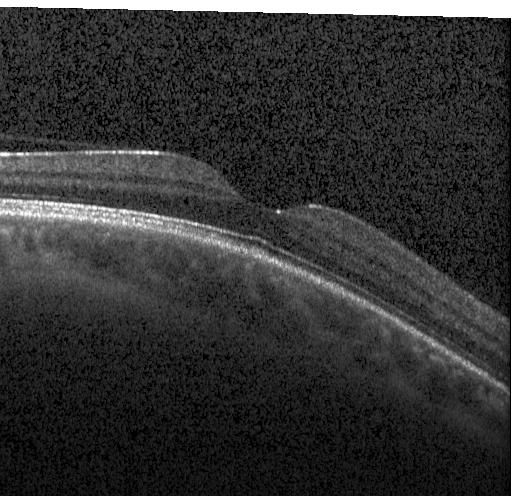
Retinal OCT B-scan — Finding: neither CNV, DME, nor drusen.